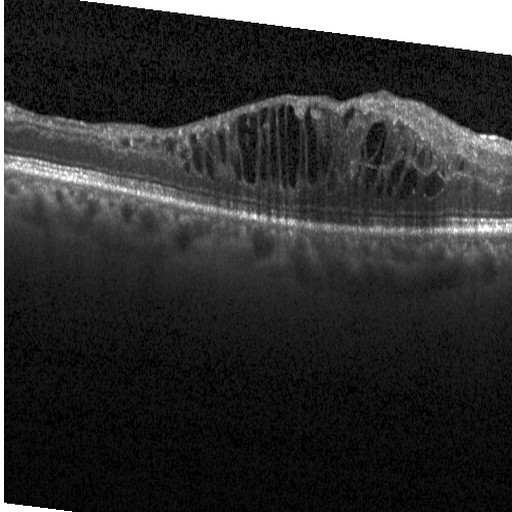
Heidelberg Spectralis, OCT B-scan.
Diagnosis: diabetic macular edema (DME).